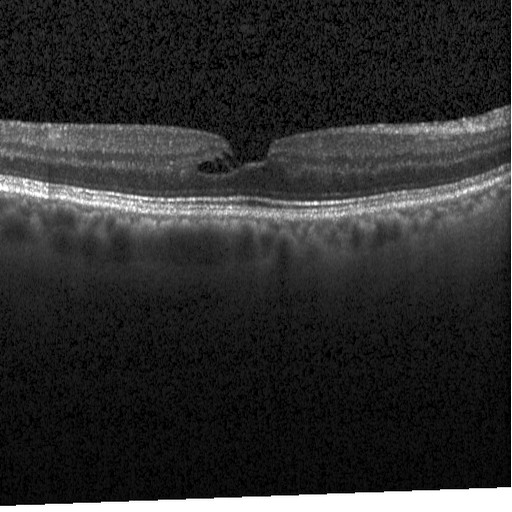
Fovea-centered · SD-OCT · OCT line scan — The scan shows diabetic macular edema.